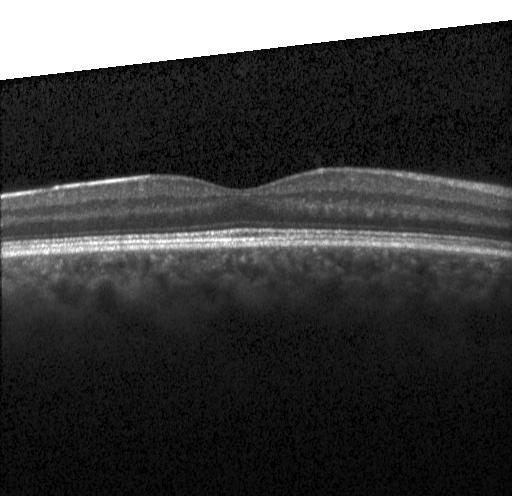 OCT B-scan showing neither CNV, DME, nor drusen.